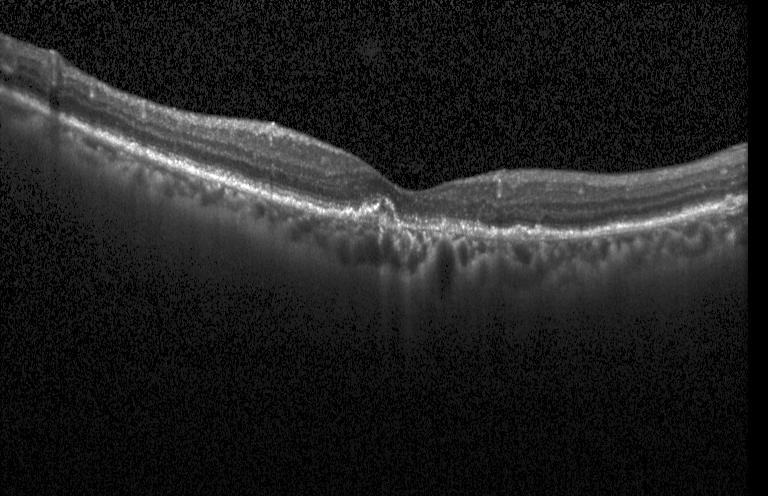 SD-OCT. OCT B-scan — A choroidal neovascular membrane.